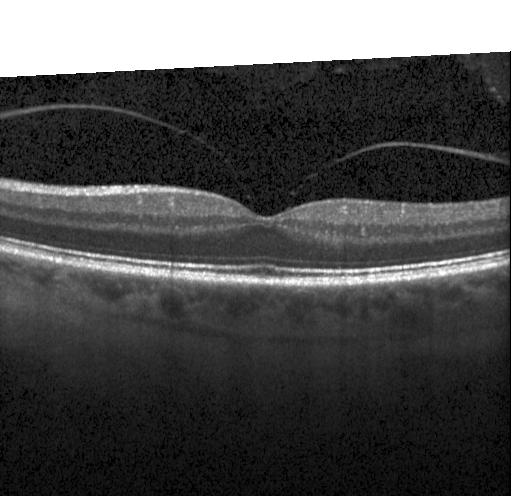

Dx: no CNV, DME, or drusen.